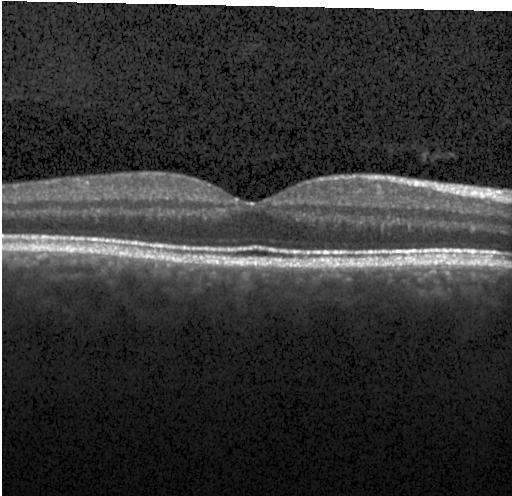

Optical coherence tomography B-scan — Dx: no evidence of choroidal neovascularization, diabetic macular edema, or drusen.